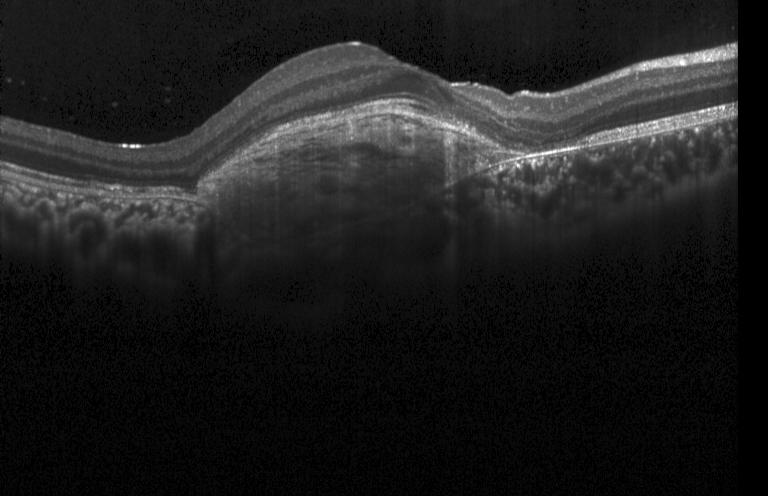

Fovea-centered. Heidelberg Spectralis. Spectral-domain OCT. Optical coherence tomography scan
This B-scan demonstrates choroidal neovascularization (CNV).